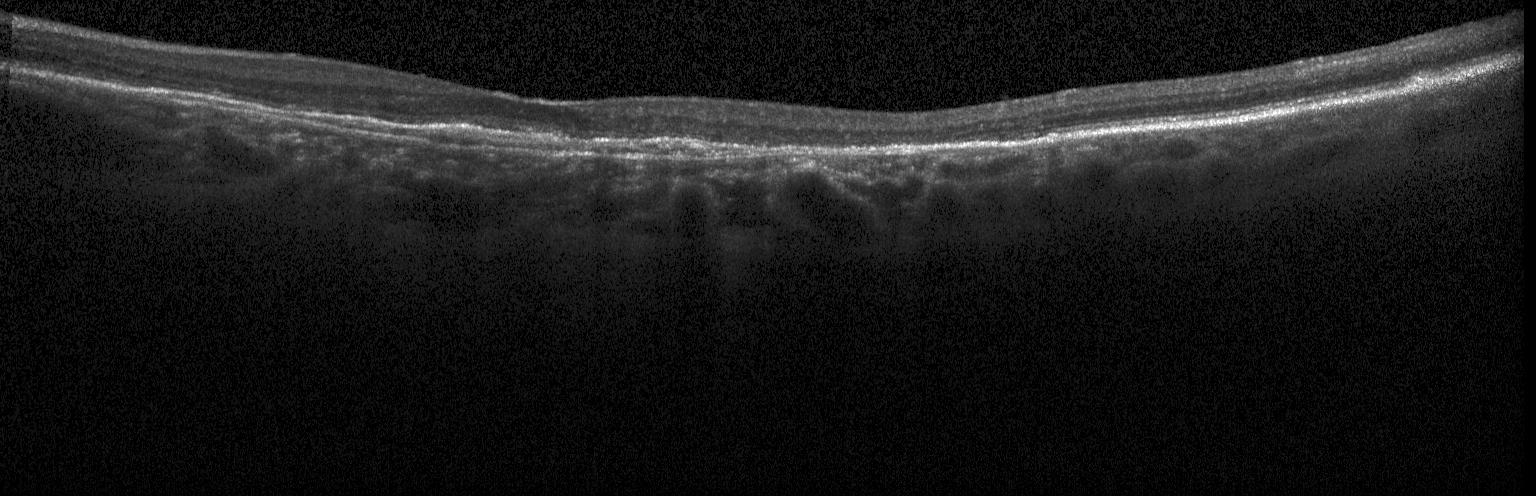

Acquired on a Heidelberg Spectralis; through the macula; optical coherence tomography B-scan.
Impression: a choroidal neovascular membrane.